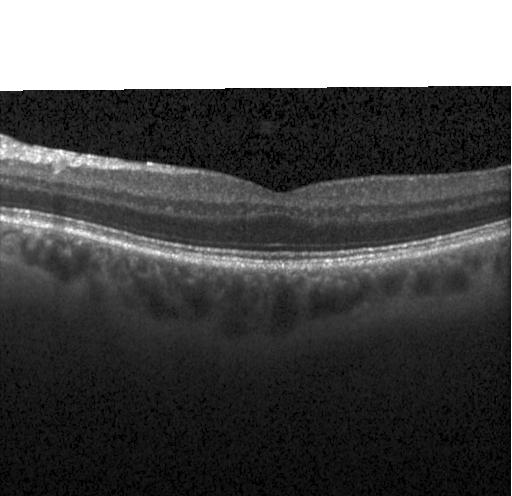
Macular OCT demonstrating neither CNV, DME, nor drusen.